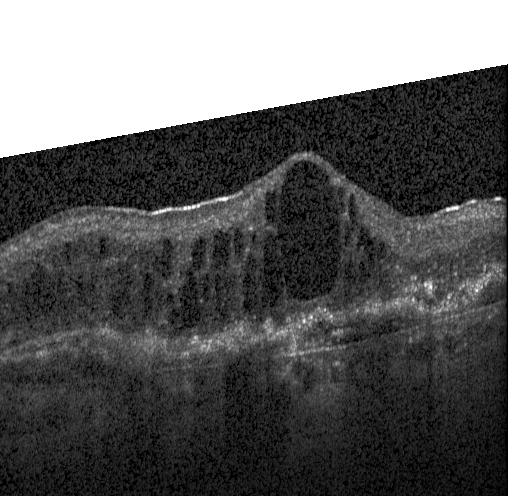

Finding: a choroidal neovascular membrane.